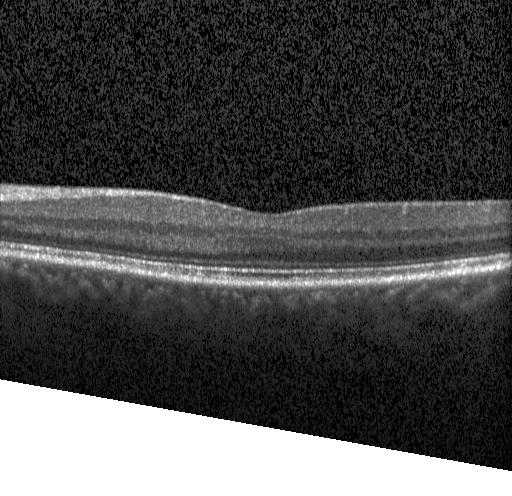

Finding: no evidence of choroidal neovascularization, diabetic macular edema, or drusen.